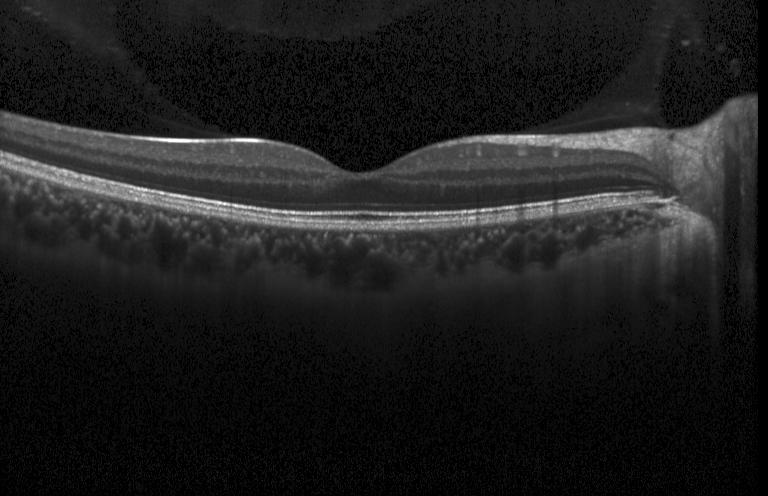
OCT B-scan showing neither CNV, DME, nor drusen.